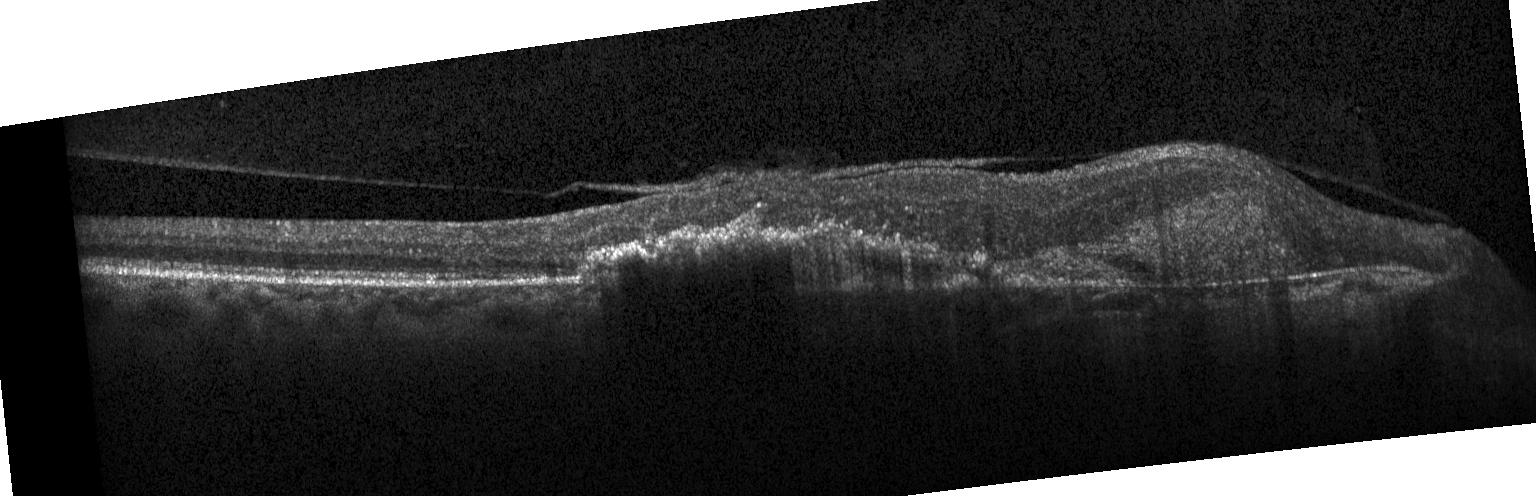
Finding: a choroidal neovascular membrane.